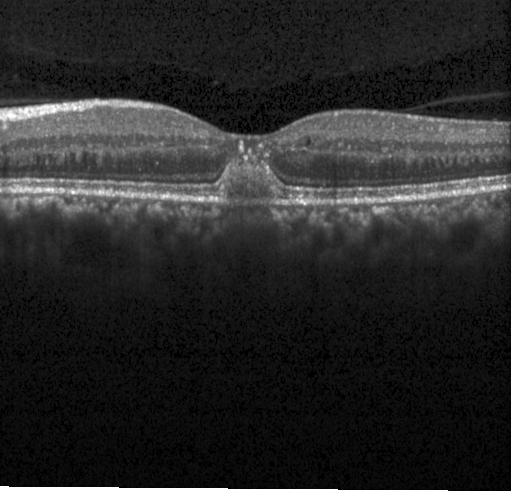 Macular OCT demonstrating choroidal neovascularization (CNV).